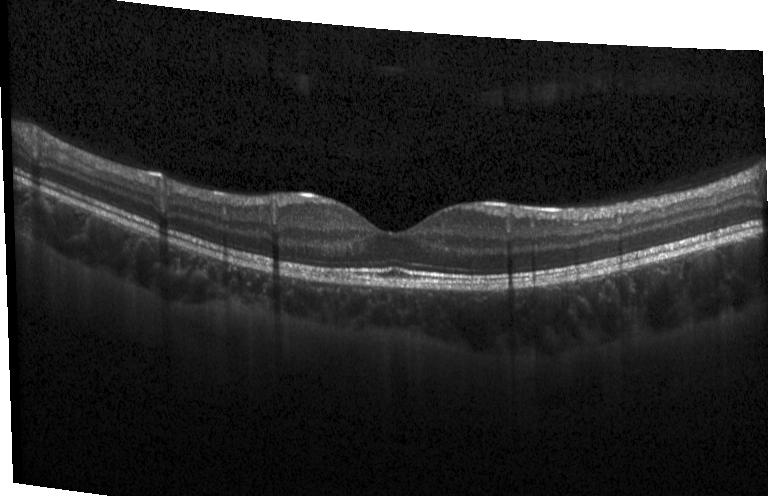

Macular scan, OCT B-scan, spectral-domain OCT
Finding: no choroidal neovascularization, no diabetic macular edema, and no drusen.